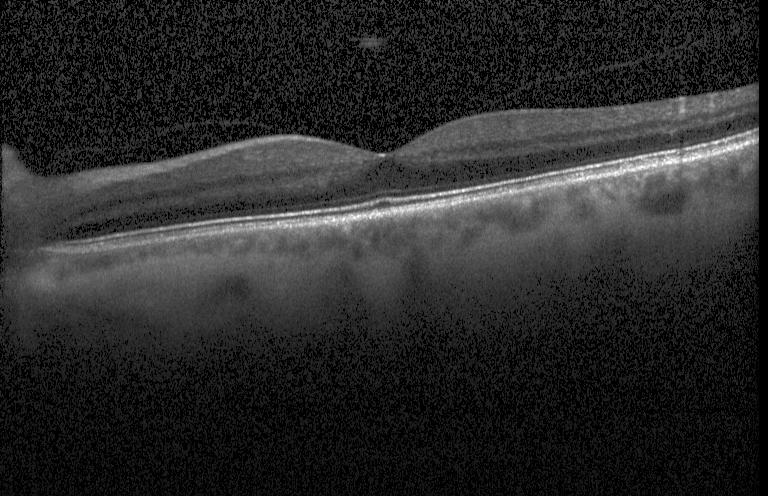

OCT B-scan, SD-OCT
Finding: neither choroidal neovascularization, diabetic macular edema, nor drusen.